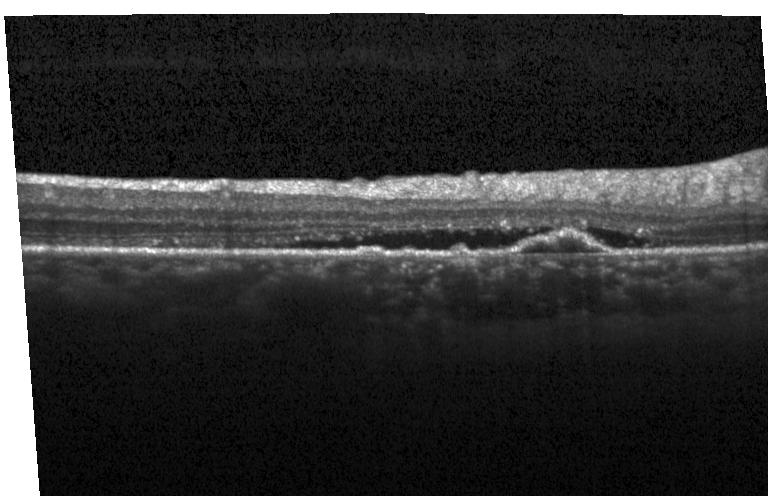 Macular scan. OCT B-scan.
This B-scan demonstrates a choroidal neovascular membrane.